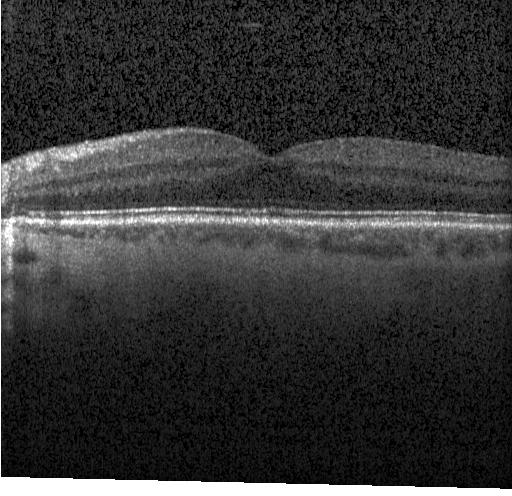

Retinal OCT cross-section · spectral-domain OCT. OCT finding: no CNV, no DME, and no drusen.